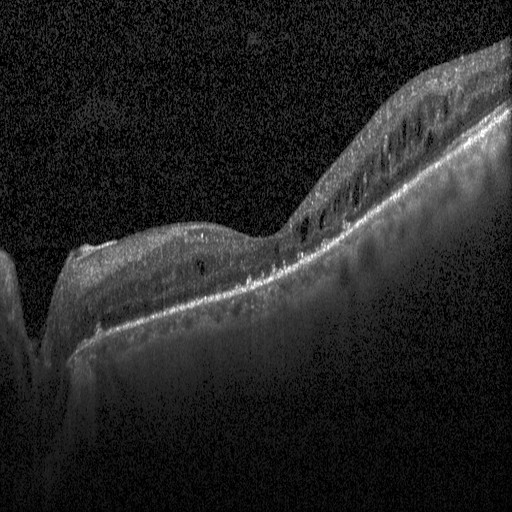 Finding: DME.